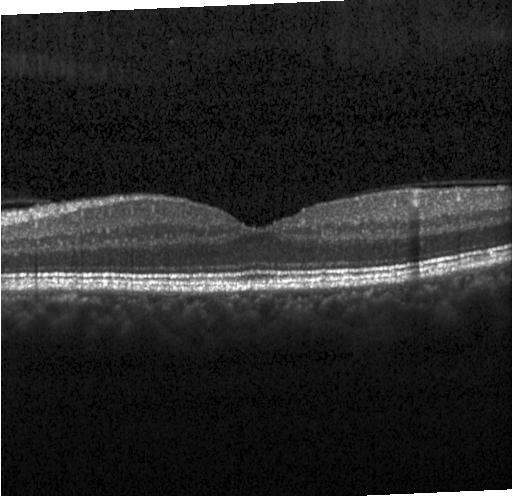
OCT line scan.
Impression: neither choroidal neovascularization, diabetic macular edema, nor drusen.